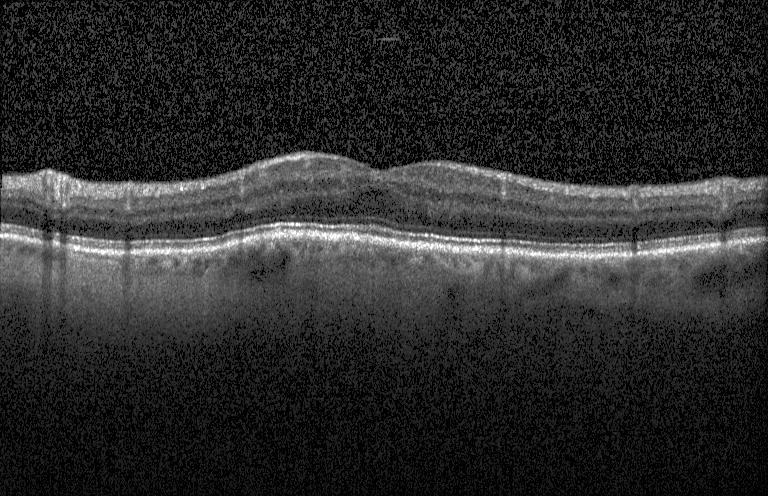
OCT finding: neither choroidal neovascularization, diabetic macular edema, nor drusen.